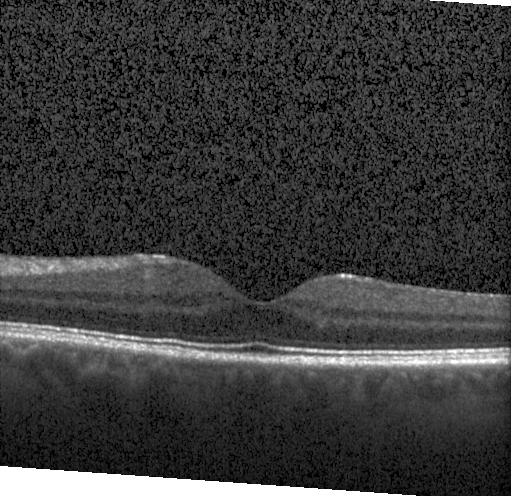 Retinal OCT cross-section, Heidelberg Spectralis OCT system, spectral-domain OCT — No CNV, DME, or drusen.